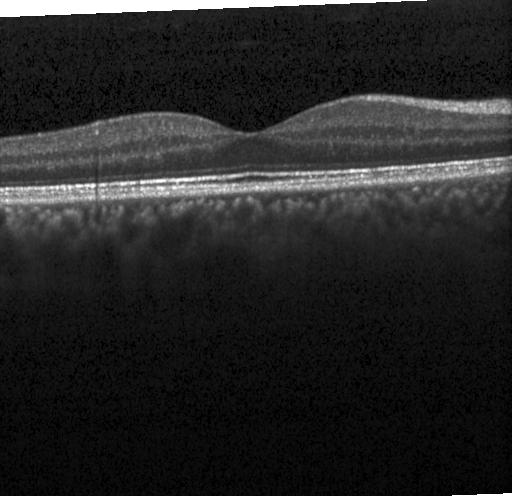
SD-OCT; macular scan; optical coherence tomography B-scan; instrument: Heidelberg Spectralis
Diagnosis: no CNV, DME, or drusen.